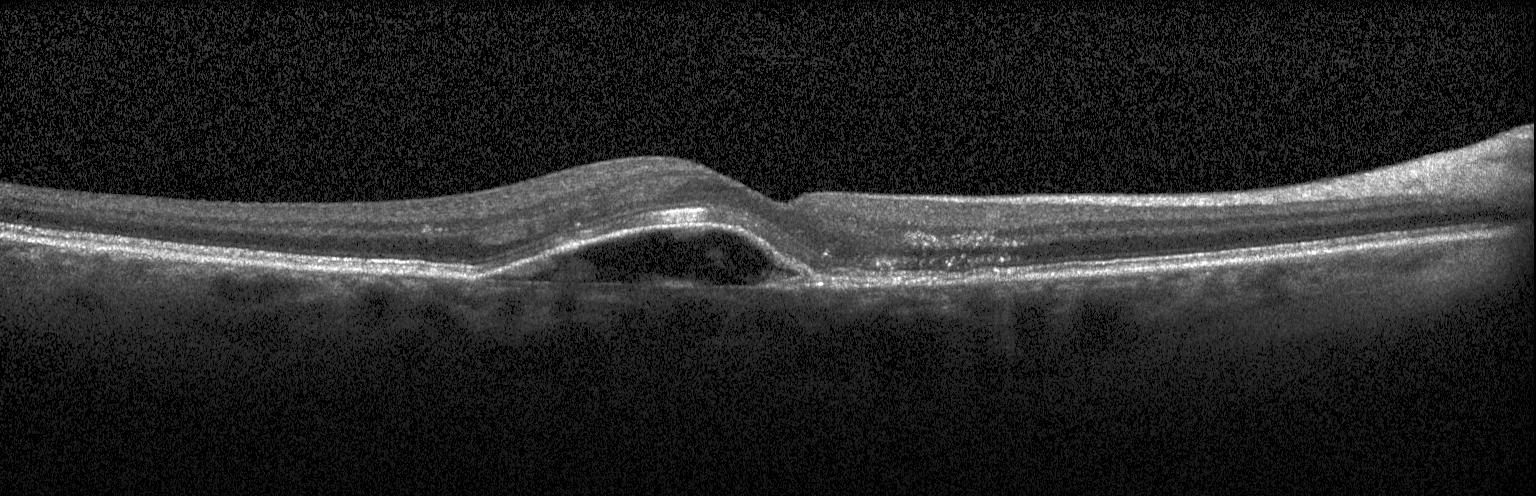
SD-OCT. Retinal OCT B-scan. Macular scan. This B-scan demonstrates a choroidal neovascular membrane.